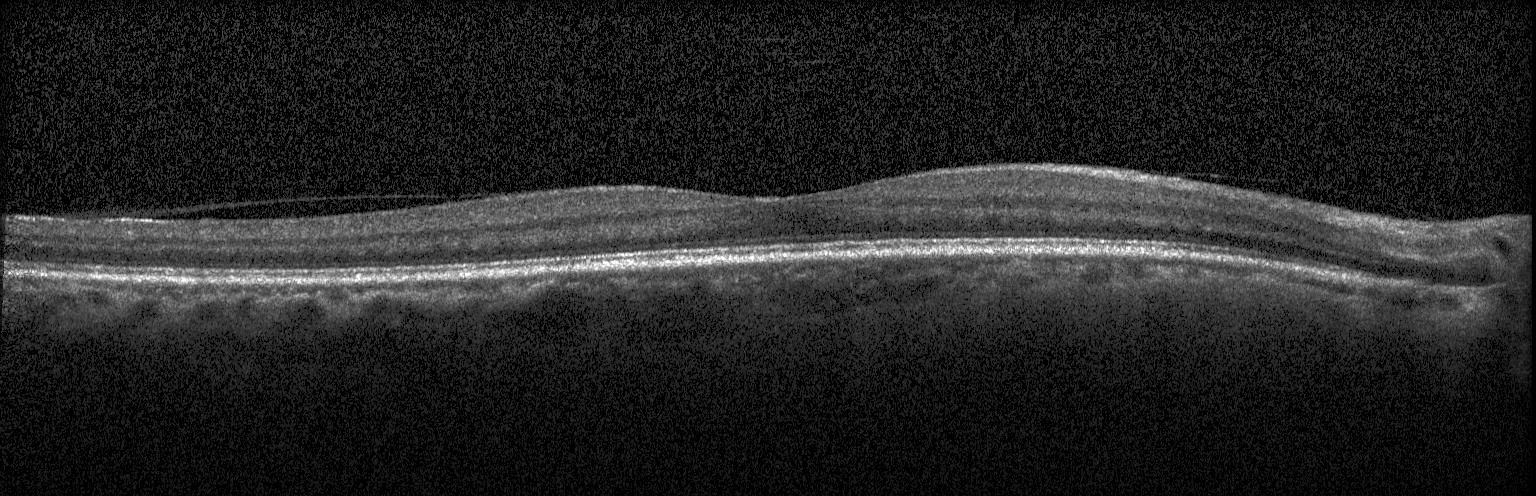 Instrument: Heidelberg Spectralis · retinal OCT cross-section · horizontal scan through the fovea
Dx: no choroidal neovascularization, no diabetic macular edema, and no drusen.